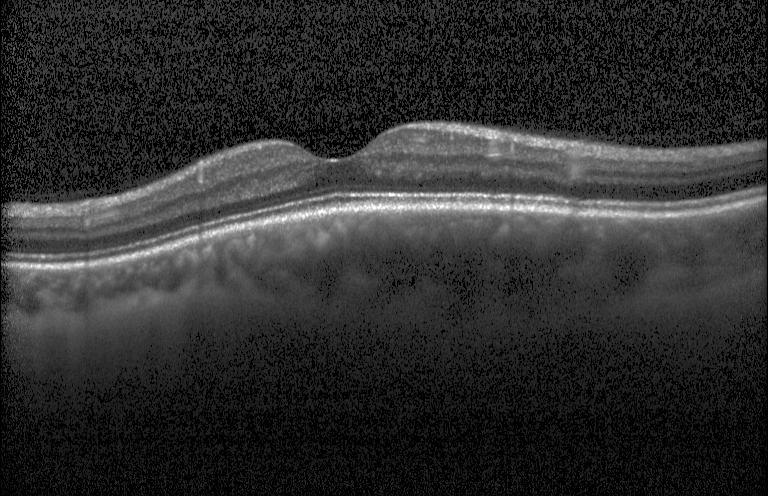

Retinal OCT cross-section · SD-OCT
This B-scan demonstrates no CNV, DME, or drusen.